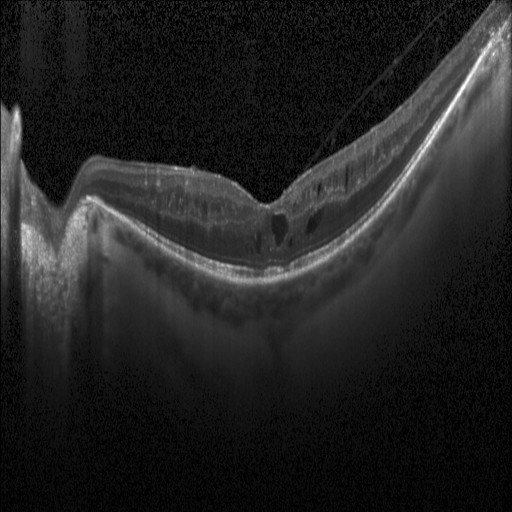
OCT scan showing DME.